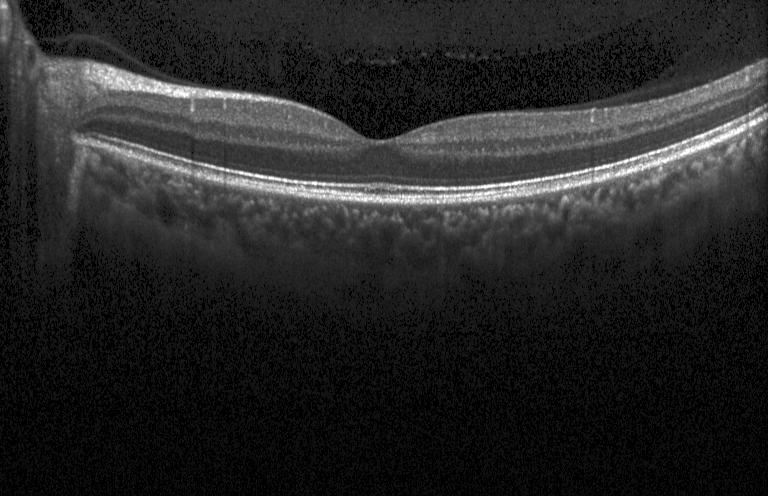
Heidelberg Spectralis · retinal OCT cross-section — OCT finding: no evidence of choroidal neovascularization, diabetic macular edema, or drusen.